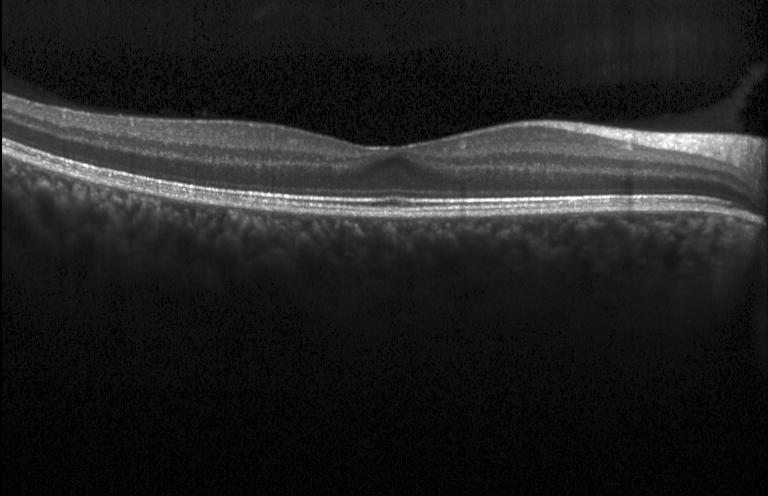

Spectral-domain optical coherence tomography. Instrument: Heidelberg Spectralis. Through the macula. Optical coherence tomography scan.
This B-scan demonstrates neither choroidal neovascularization, diabetic macular edema, nor drusen.